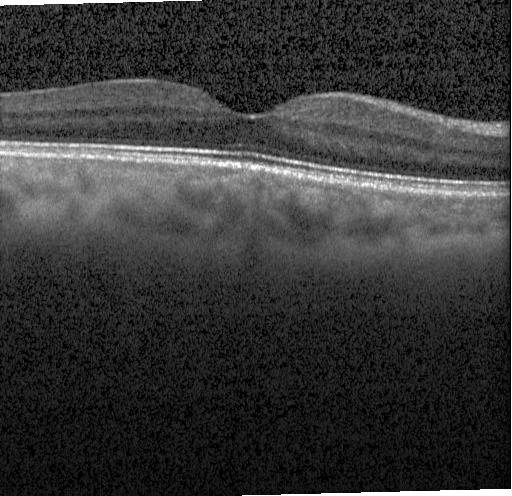
Spectral-domain OCT · centered on the fovea · retinal OCT B-scan. Diagnosis: neither choroidal neovascularization, diabetic macular edema, nor drusen.